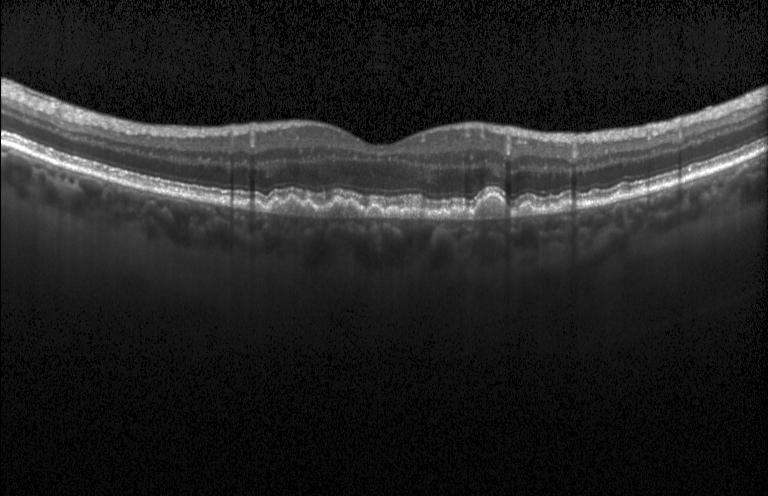

Fovea-centered · retinal OCT B-scan.
Multiple drusen.